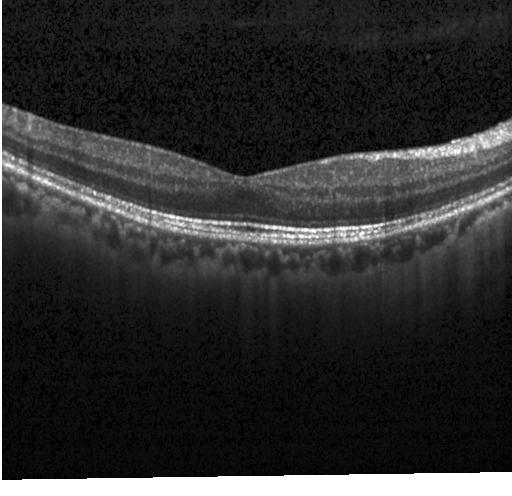
Finding: no evidence of choroidal neovascularization, diabetic macular edema, or drusen.